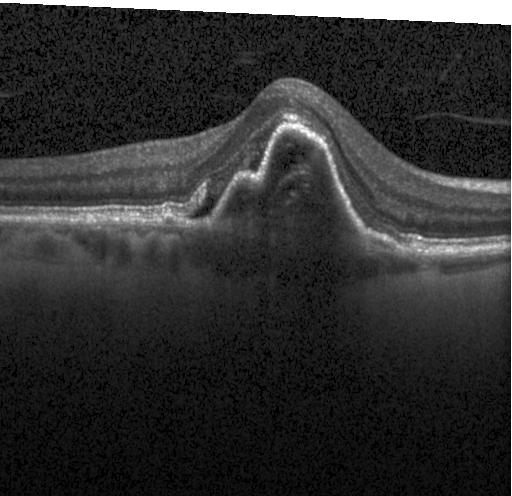 Retinal OCT B-scan; centered on the fovea.
Impression: choroidal neovascularization.